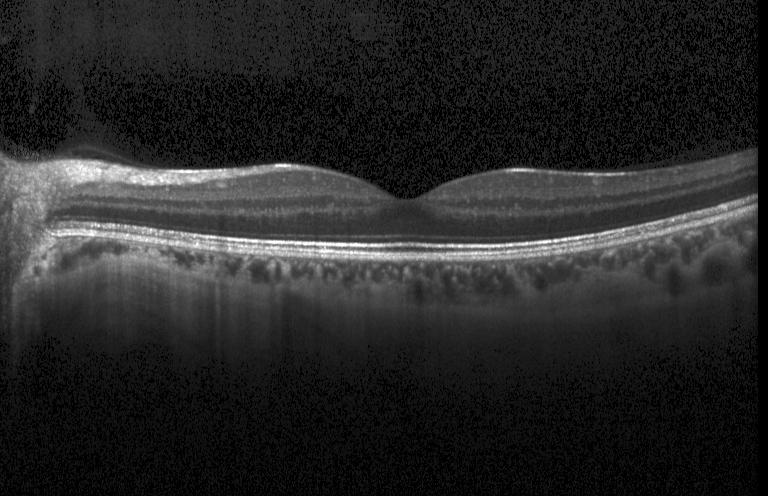

Assessment: neither choroidal neovascularization, diabetic macular edema, nor drusen.